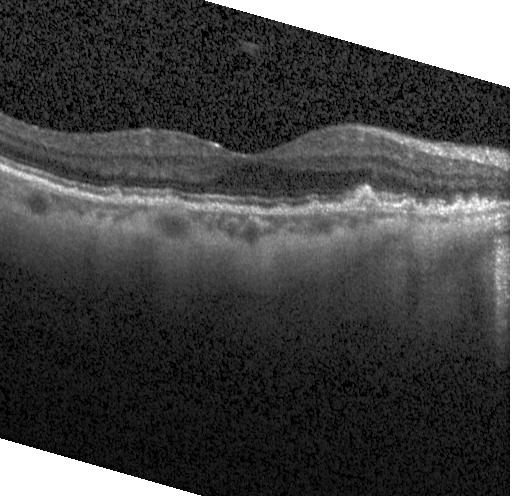

Impression: multiple drusen.